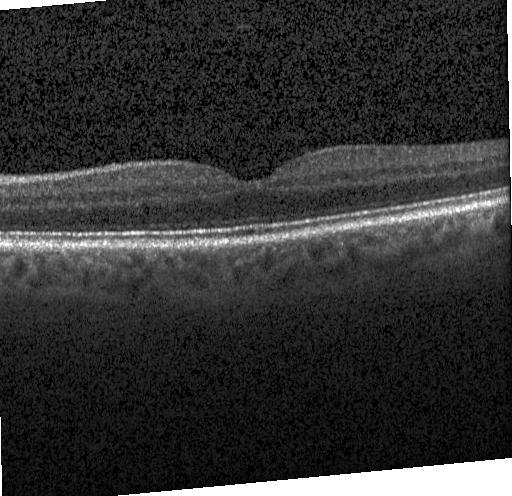

Macular OCT demonstrating no evidence of choroidal neovascularization, diabetic macular edema, or drusen.